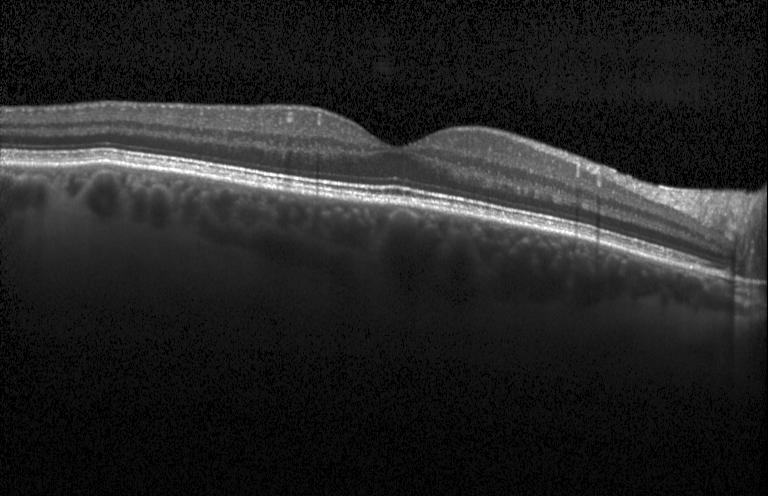 Spectral-domain OCT, through the macula, OCT B-scan.
Assessment: no choroidal neovascularization, no diabetic macular edema, and no drusen.